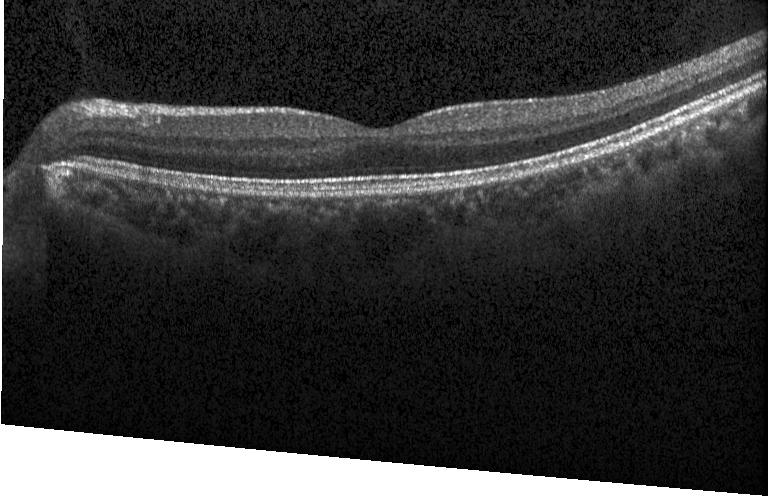 Instrument: Heidelberg Spectralis, retinal OCT B-scan. Dx: no choroidal neovascularization, no diabetic macular edema, and no drusen.